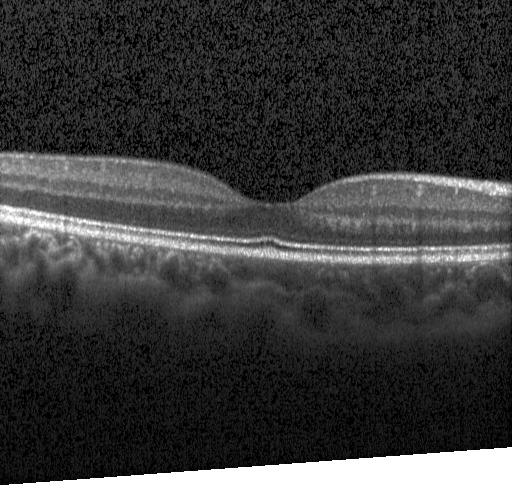

Macular scan, OCT line scan, spectral-domain optical coherence tomography — Macular OCT: neither choroidal neovascularization, diabetic macular edema, nor drusen.